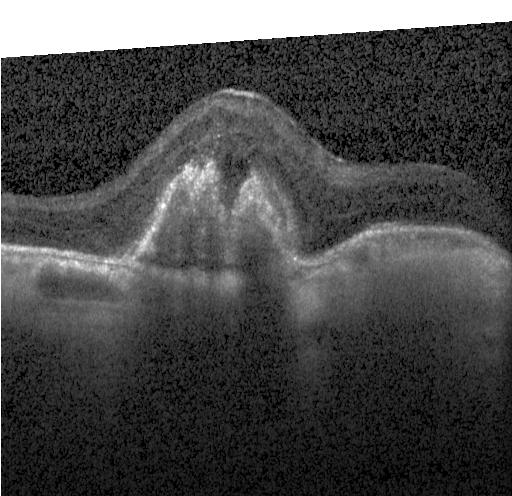
Retinal OCT B-scan. Assessment: a choroidal neovascular membrane.